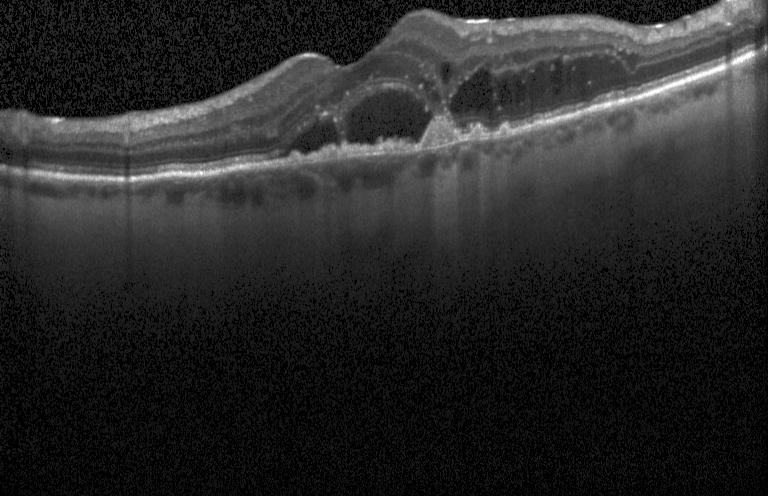
Heidelberg Spectralis; spectral-domain optical coherence tomography; OCT line scan. Dx: a choroidal neovascular membrane.